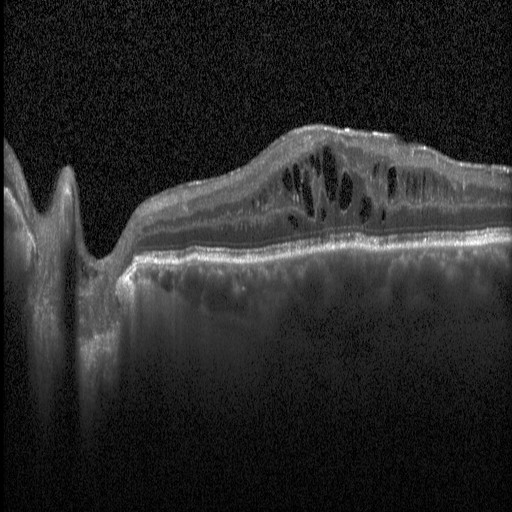

OCT finding: DME.